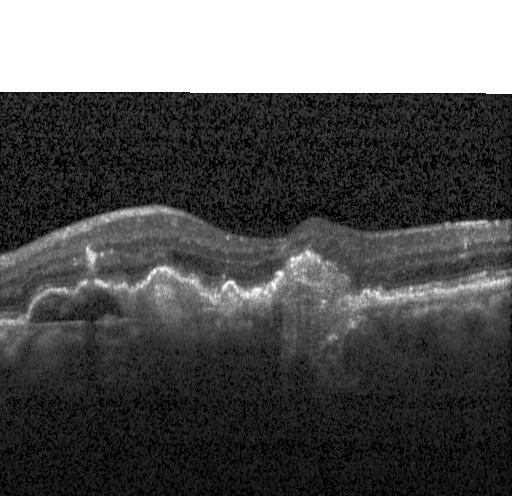

Impression: a choroidal neovascular membrane.